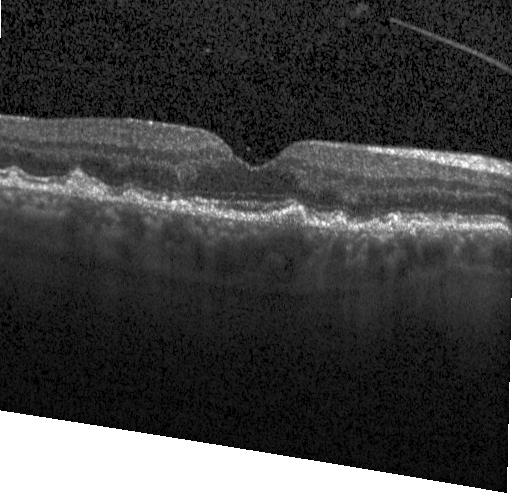 Retinal OCT cross-section showing drusen.